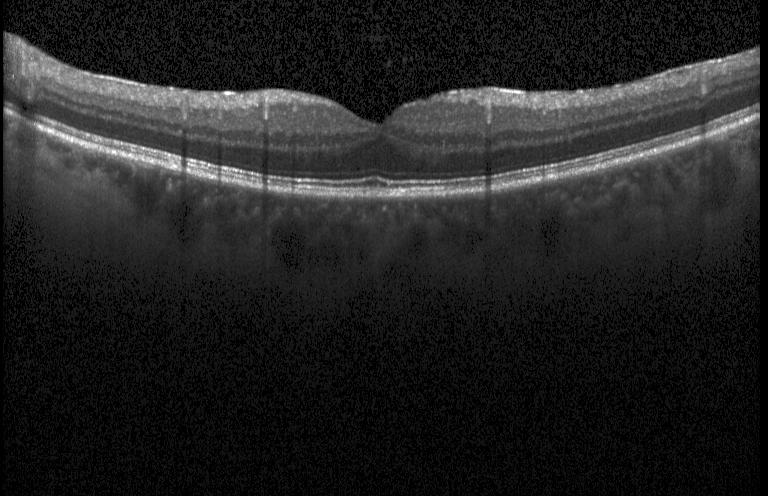

Diagnosis: no CNV, no DME, and no drusen.